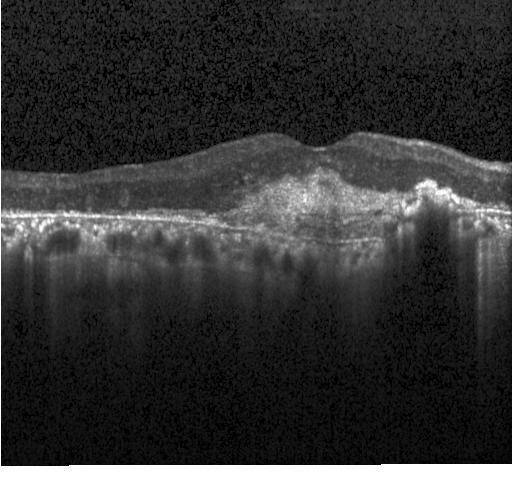

Spectral-domain optical coherence tomography · OCT B-scan · Heidelberg Spectralis OCT system · through the macula — Assessment: a choroidal neovascular membrane.